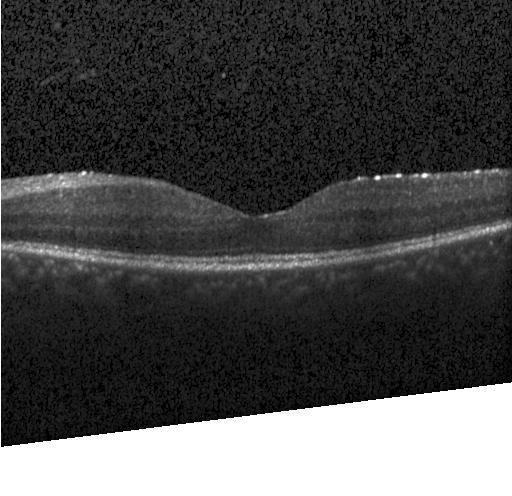

Optical coherence tomography B-scan — Macular OCT: no evidence of choroidal neovascularization, diabetic macular edema, or drusen.